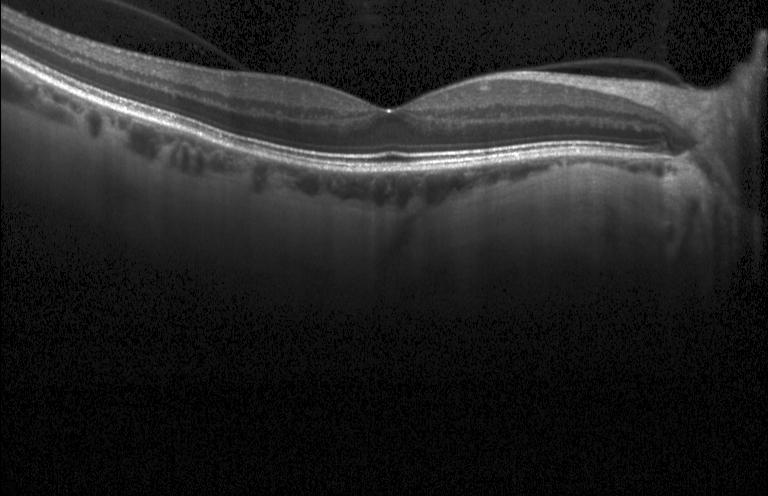
Heidelberg Spectralis OCT system · retinal OCT cross-section · fovea-centered. OCT finding: neither CNV, DME, nor drusen.